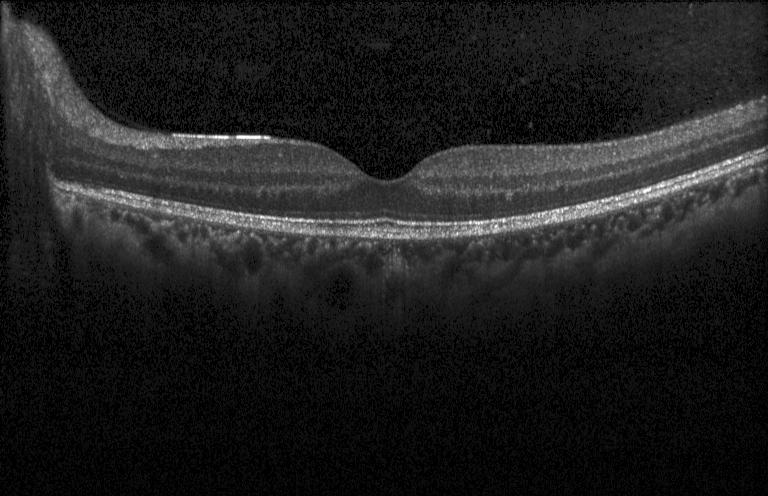
Heidelberg Spectralis OCT system, SD-OCT, OCT line scan
Assessment: no choroidal neovascularization, diabetic macular edema, or drusen.